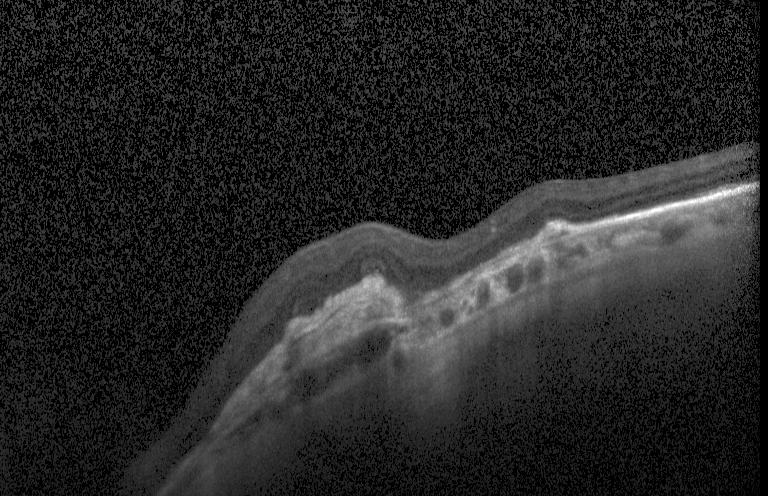 OCT finding: CNV.